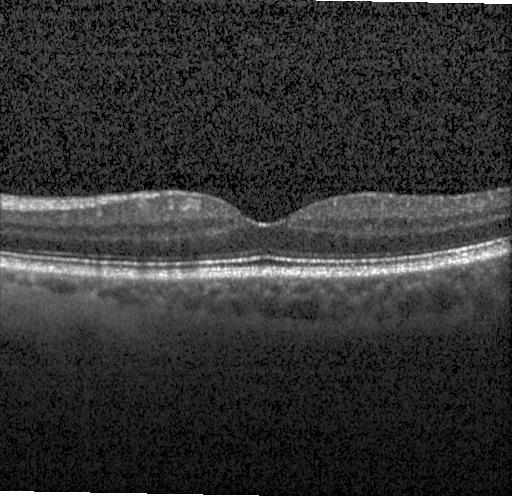
Acquired on a Heidelberg Spectralis · spectral-domain OCT · OCT line scan · centered on the fovea.
OCT finding: neither choroidal neovascularization, diabetic macular edema, nor drusen.